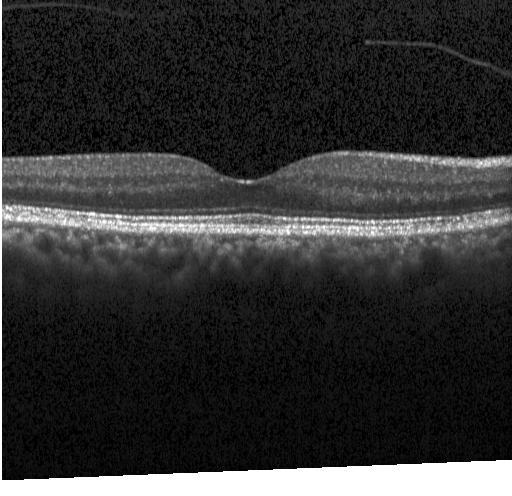
Finding: no CNV, no DME, and no drusen.